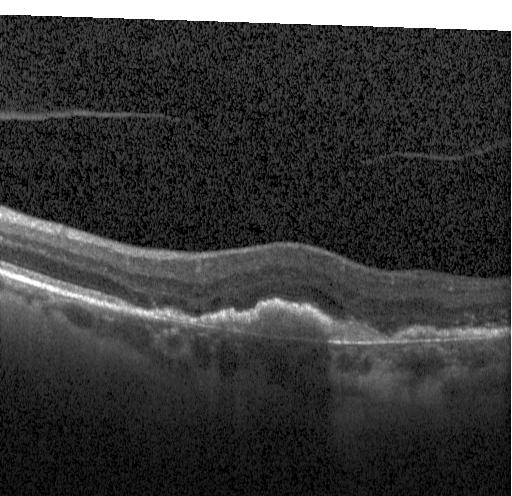
Finding: a choroidal neovascular membrane.